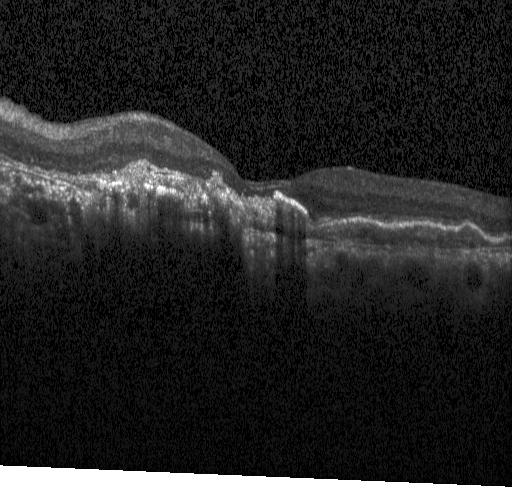
Retinal OCT B-scan — Dx: choroidal neovascularization (CNV).